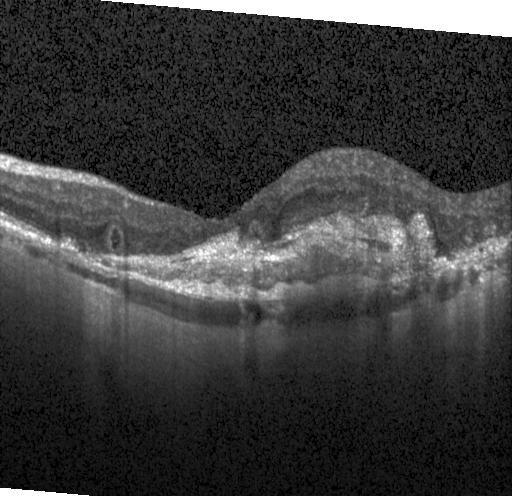 OCT finding: a choroidal neovascular membrane.